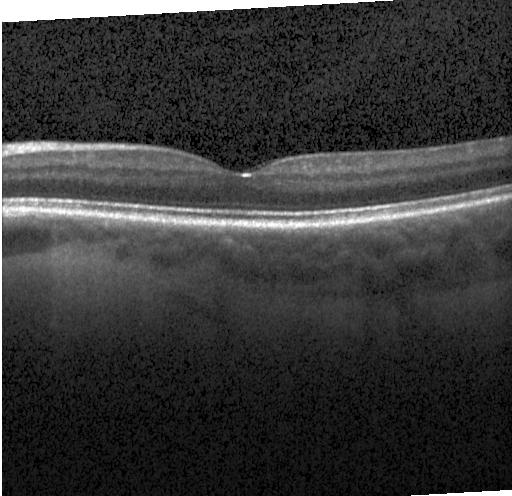
Horizontal scan through the fovea. Optical coherence tomography scan.
Assessment: no evidence of choroidal neovascularization, diabetic macular edema, or drusen.